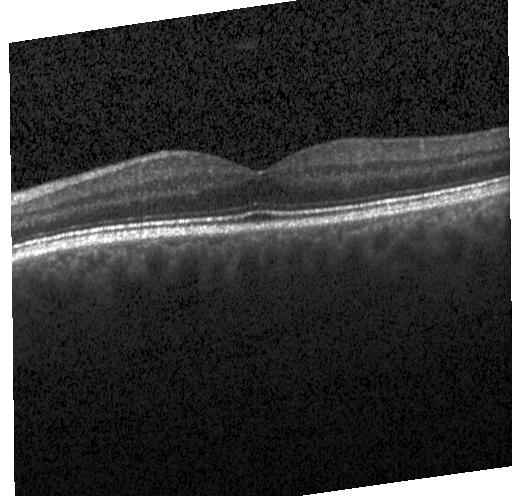 Instrument: Heidelberg Spectralis, retinal OCT B-scan, SD-OCT — The scan shows no choroidal neovascularization, diabetic macular edema, or drusen.